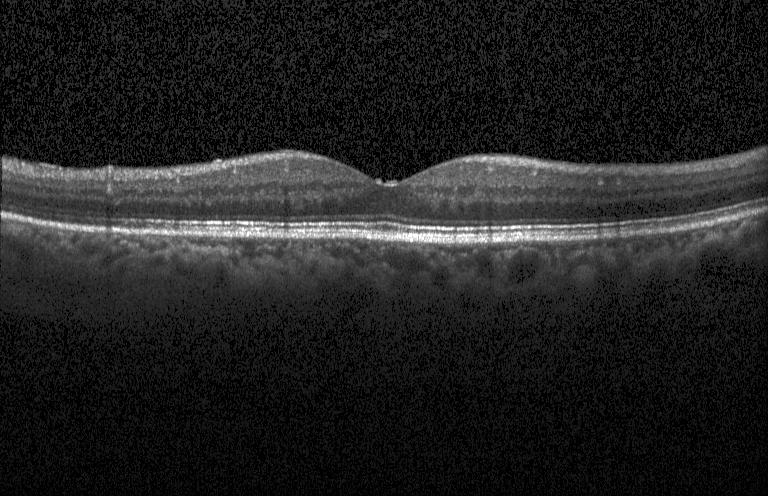
OCT scan showing no CNV, DME, or drusen.